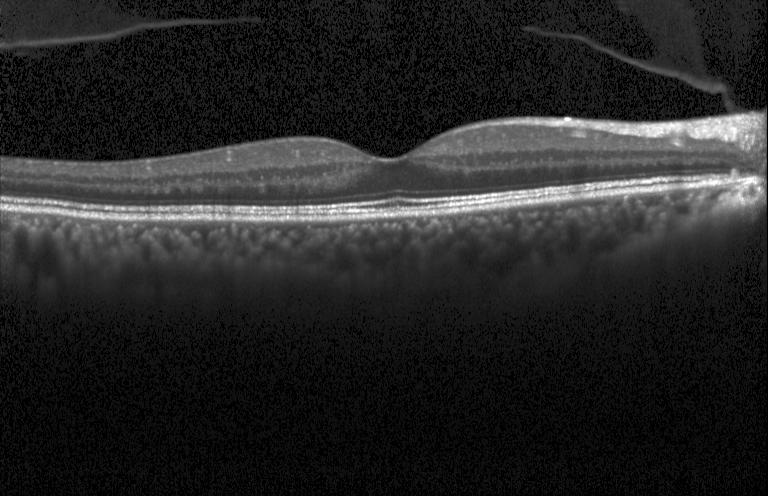

Instrument: Heidelberg Spectralis. Fovea-centered. Spectral-domain optical coherence tomography. Optical coherence tomography B-scan. OCT finding: no CNV, no DME, and no drusen.